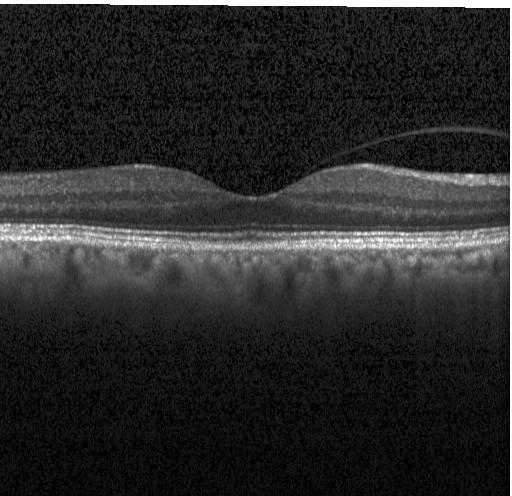
Diagnosis: no choroidal neovascularization, diabetic macular edema, or drusen.